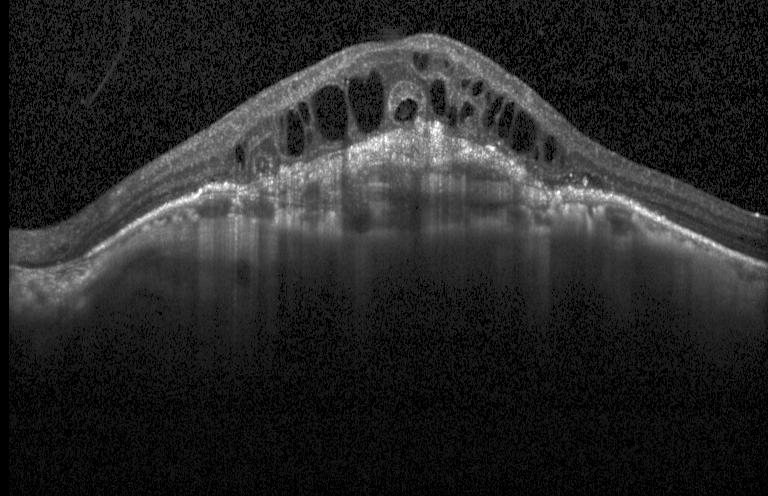

Retinal OCT cross-section. Heidelberg Spectralis. Through the macula. SD-OCT.
This B-scan demonstrates CNV.